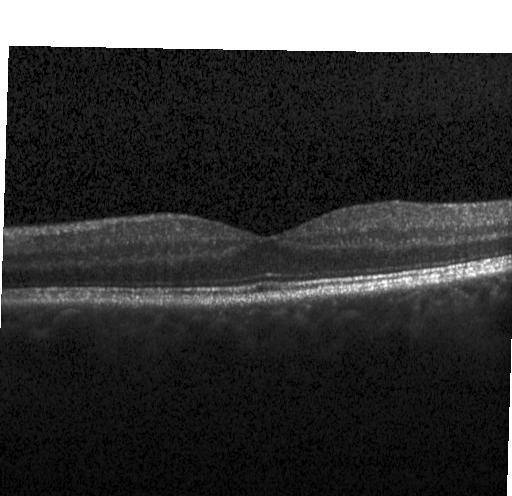
Dx: no choroidal neovascularization, diabetic macular edema, or drusen.